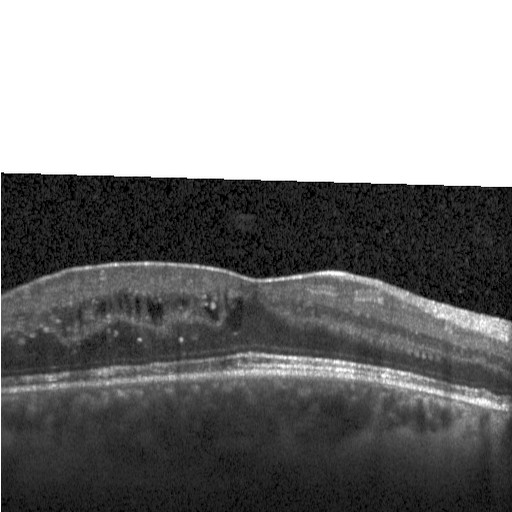 Impression: diabetic macular edema.